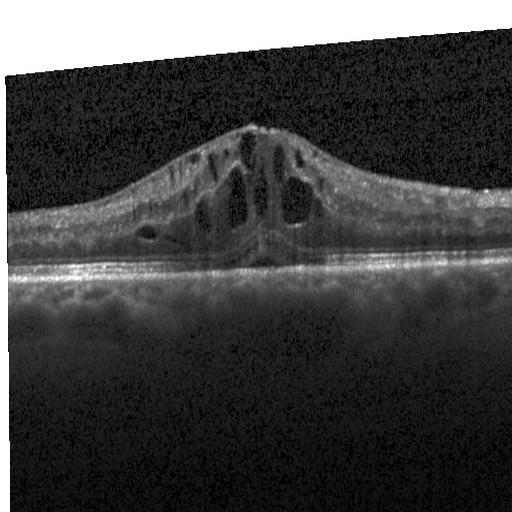

Macular OCT: diabetic macular edema.